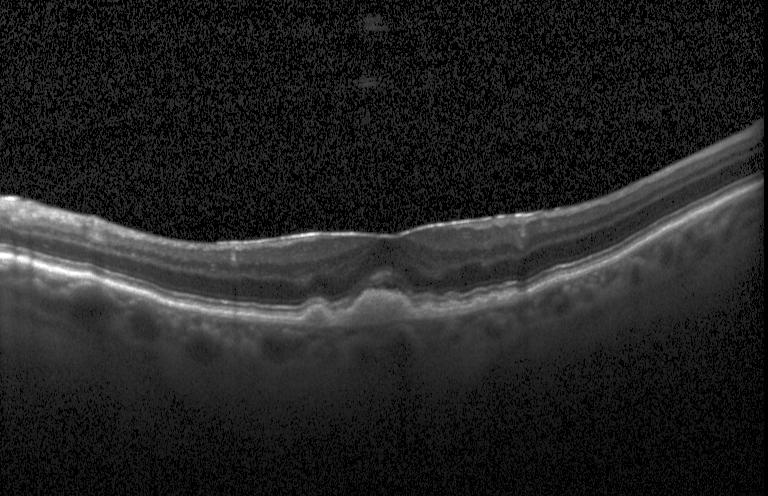
Finding: multiple drusen.